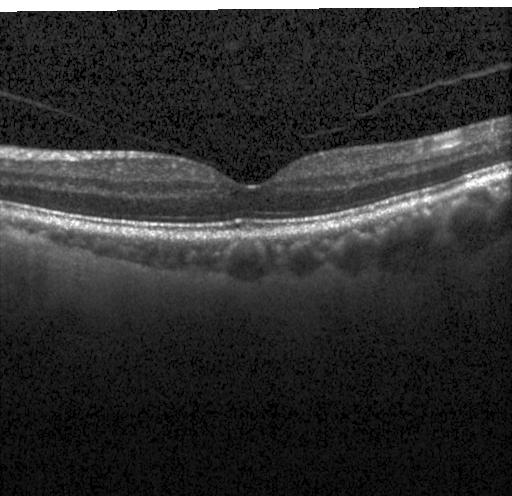
Heidelberg Spectralis, spectral-domain OCT, OCT line scan, fovea-centered — Impression: no CNV, no DME, and no drusen.